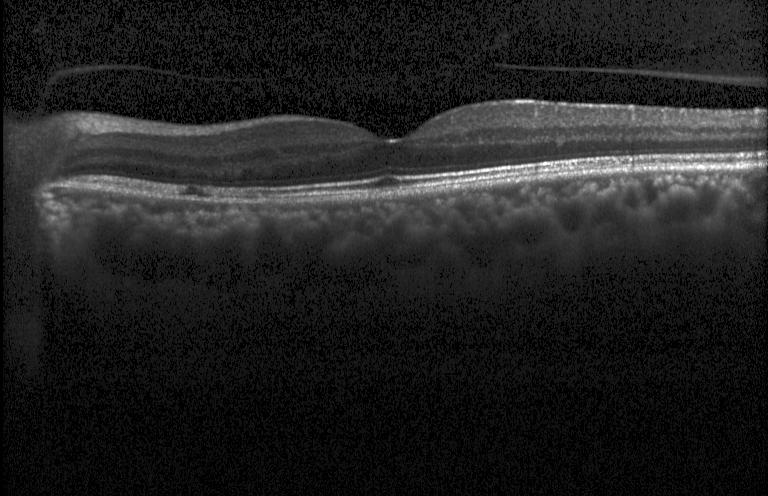

Retinal OCT cross-section showing no choroidal neovascularization, no diabetic macular edema, and no drusen.